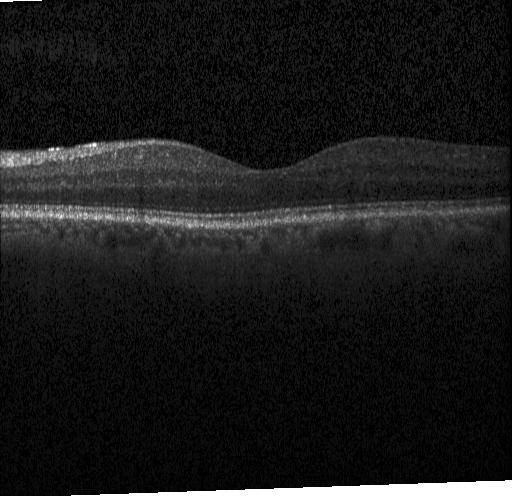

Retinal OCT B-scan. This B-scan demonstrates no CNV, no DME, and no drusen.